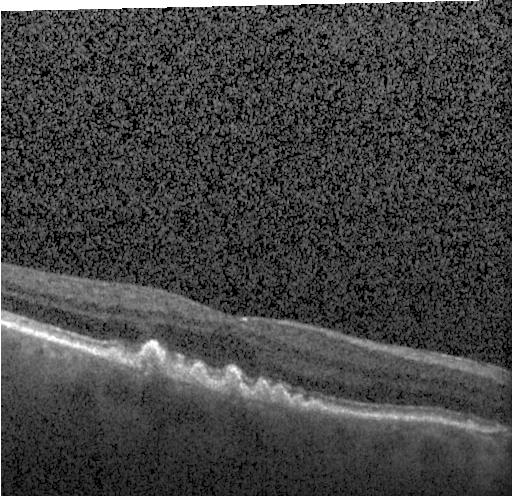
Finding: multiple drusen.